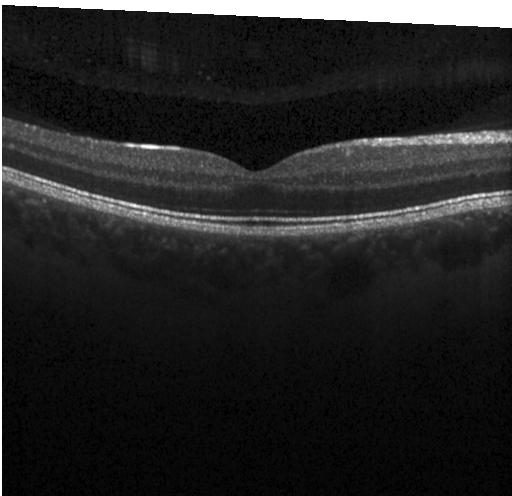 Heidelberg Spectralis, OCT B-scan, through the macula
No choroidal neovascularization, no diabetic macular edema, and no drusen.